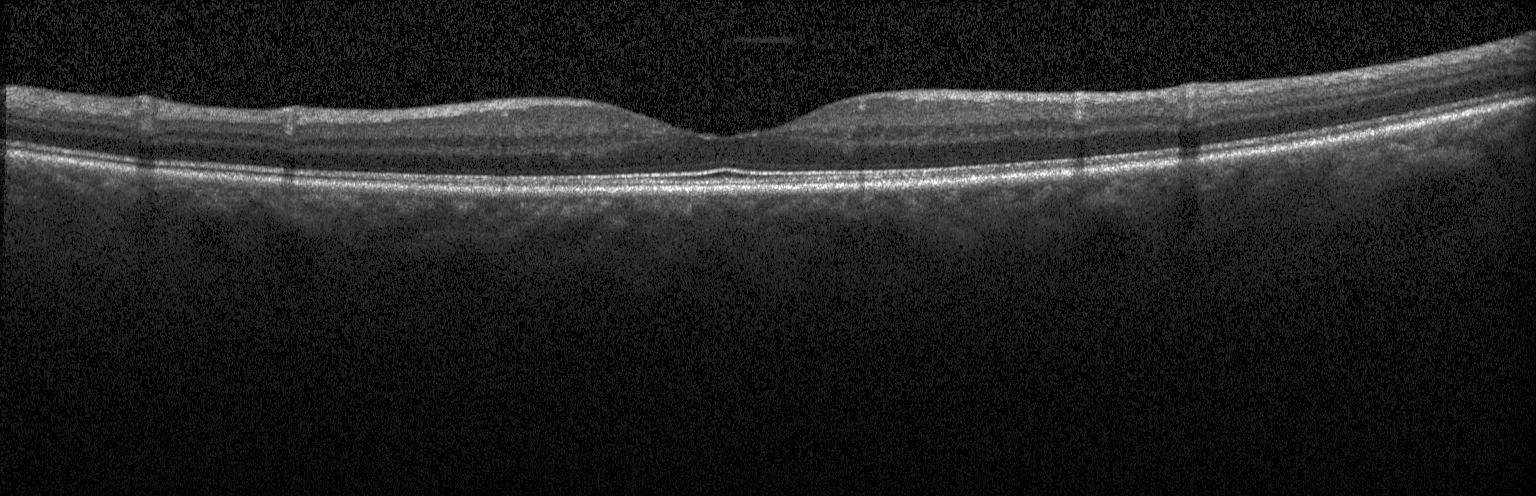

Retinal OCT B-scan, macular scan, Heidelberg Spectralis, spectral-domain OCT — Impression: no choroidal neovascularization, no diabetic macular edema, and no drusen.